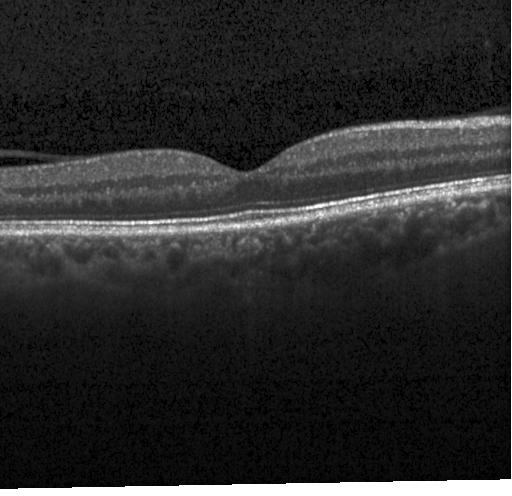
Horizontal scan through the fovea; retinal OCT B-scan — Dx: no evidence of choroidal neovascularization, diabetic macular edema, or drusen.